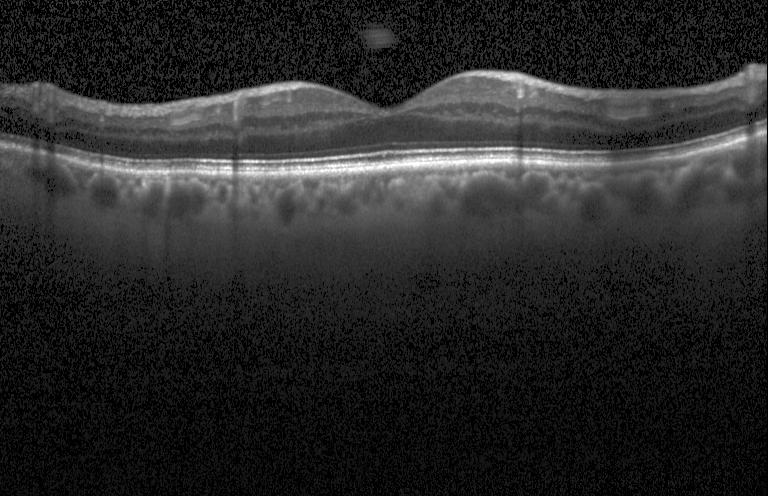 SD-OCT; OCT B-scan; instrument: Heidelberg Spectralis — The scan shows no CNV, DME, or drusen.